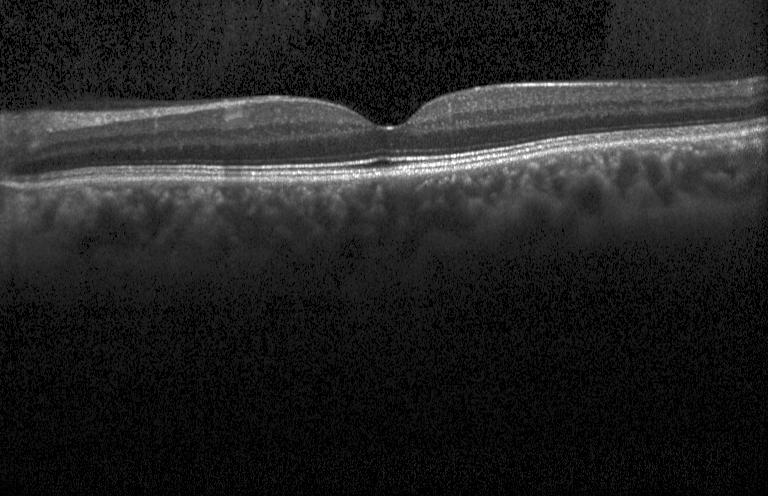 Retinal OCT cross-section showing no CNV, DME, or drusen.